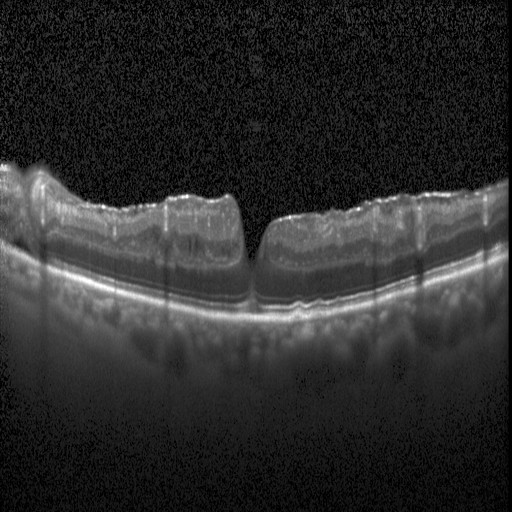
Heidelberg Spectralis; retinal OCT B-scan — The scan shows DME.